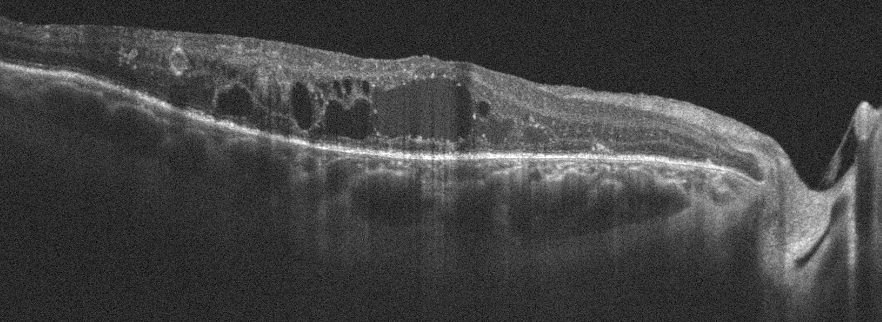
Acquired on an Optovue Avanti RTVue XR · OCT line scan.
OCT finding: DME.